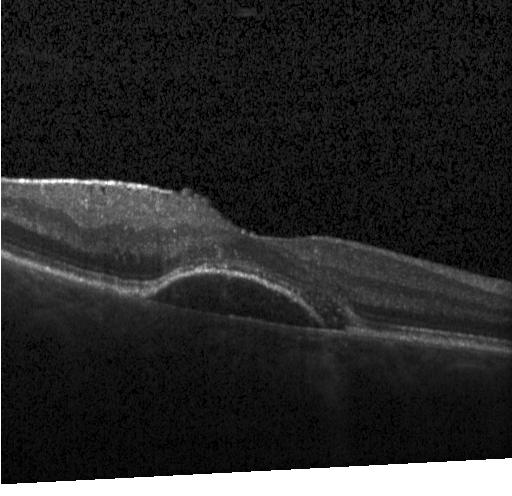

Through the macula · OCT line scan — Finding: a choroidal neovascular membrane.